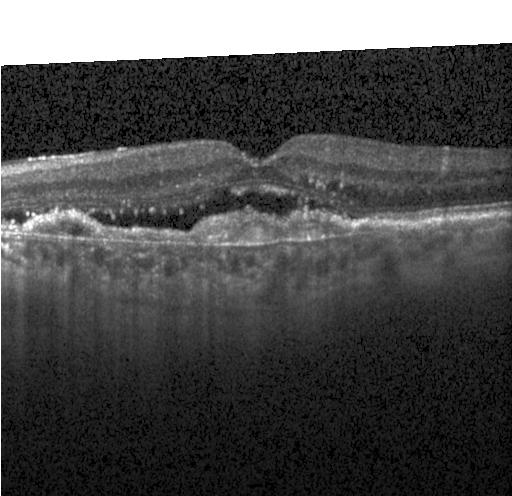 Spectral-domain optical coherence tomography; optical coherence tomography B-scan
Impression: choroidal neovascularization.